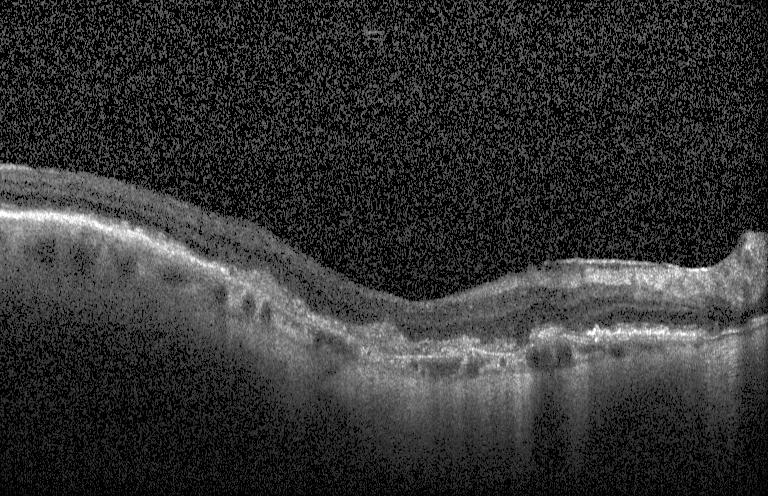

Impression: a choroidal neovascular membrane.